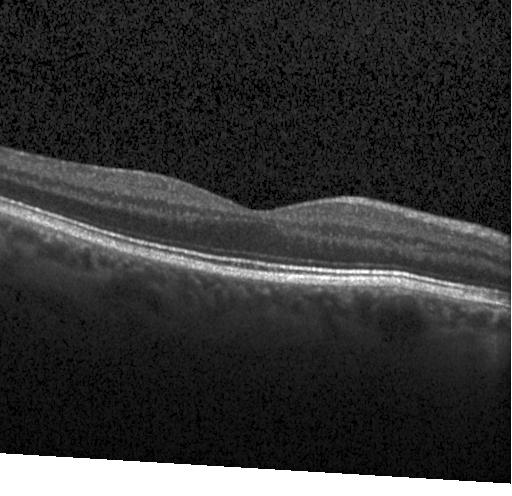
OCT line scan.
No choroidal neovascularization, no diabetic macular edema, and no drusen.